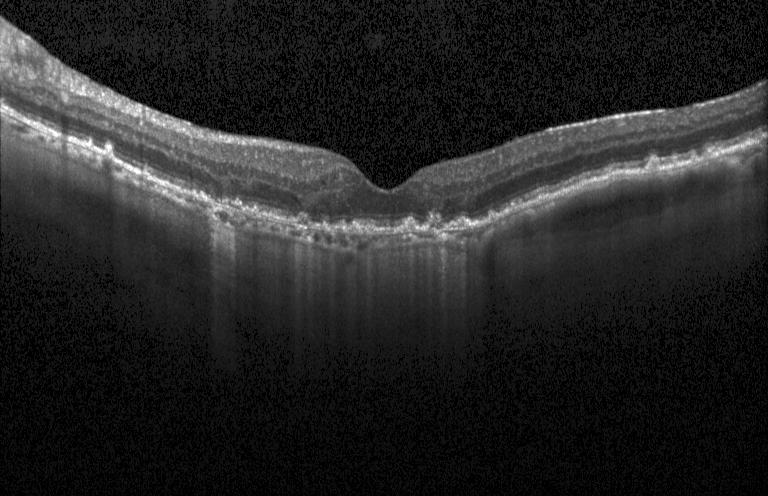

Spectral-domain OCT. Retinal OCT cross-section. Fovea-centered
Diagnosis: a choroidal neovascular membrane.